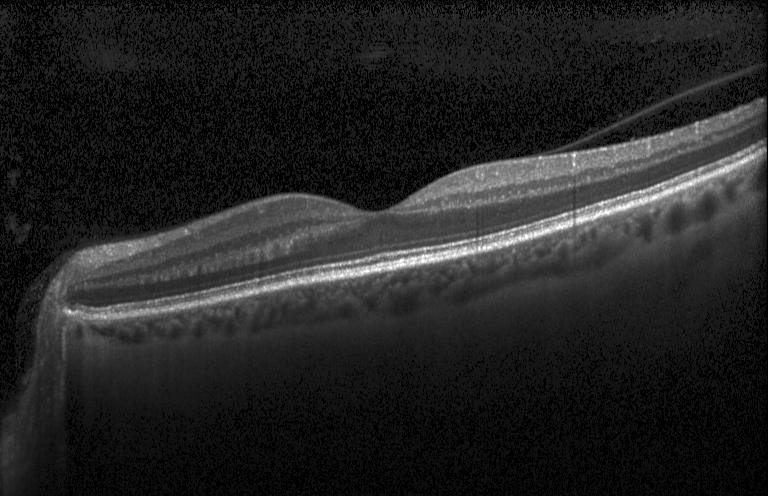 Diagnosis: neither choroidal neovascularization, diabetic macular edema, nor drusen.